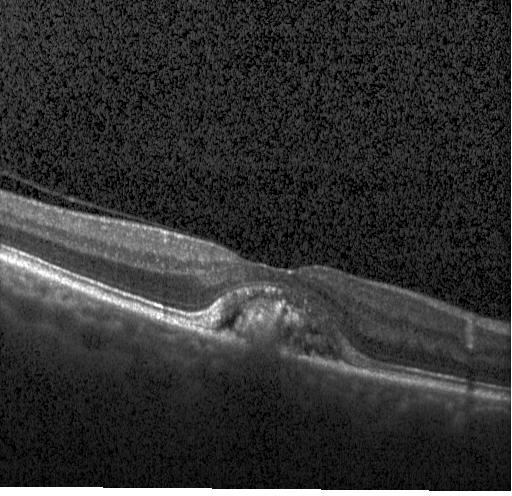

Horizontal scan through the fovea · instrument: Heidelberg Spectralis · retinal OCT B-scan — This B-scan demonstrates CNV.